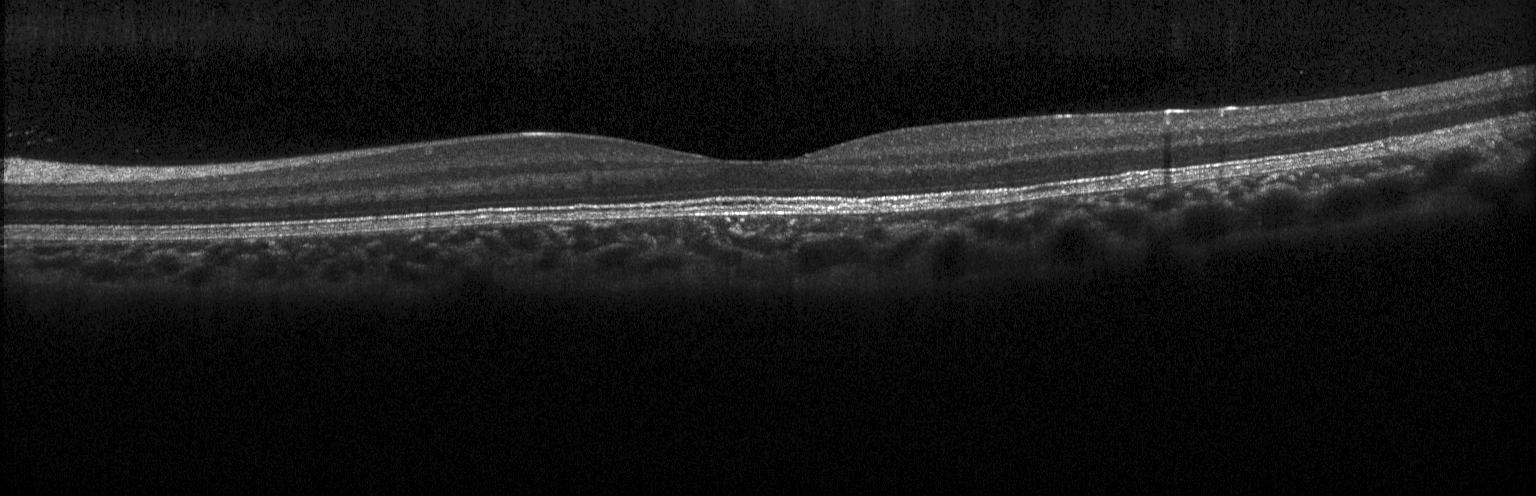
Optical coherence tomography B-scan
Impression: no choroidal neovascularization, no diabetic macular edema, and no drusen.